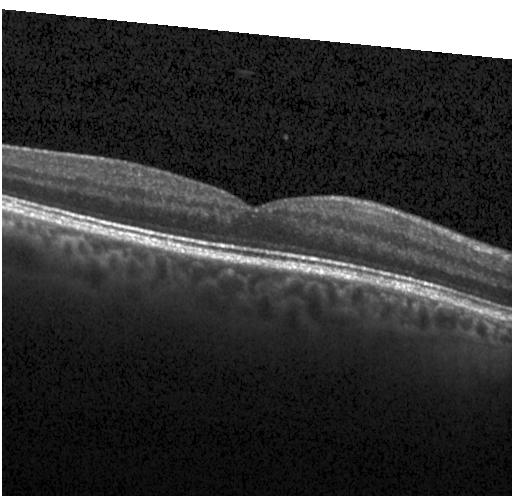

Retinal OCT cross-section
Dx: no CNV, no DME, and no drusen.